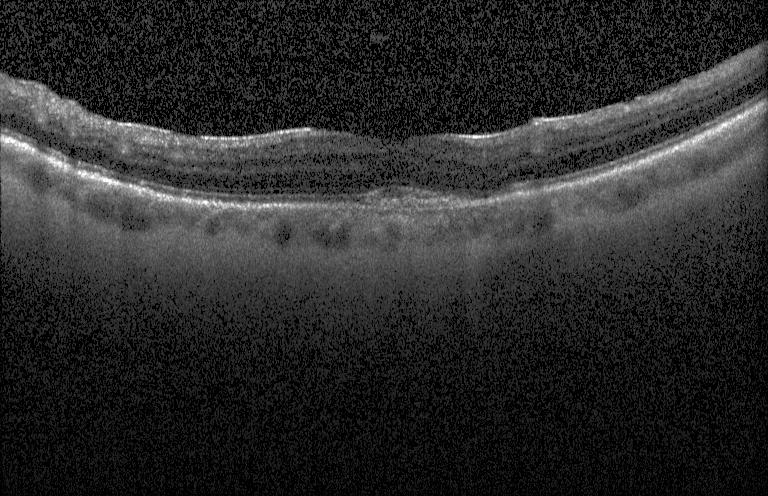
Heidelberg Spectralis · optical coherence tomography scan · centered on the fovea — Finding: choroidal neovascularization.